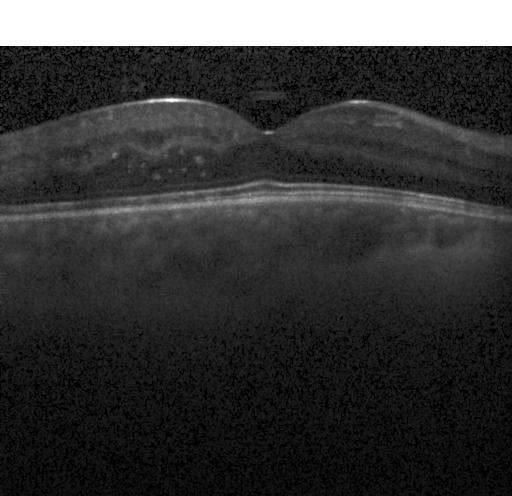

Spectral-domain optical coherence tomography · retinal OCT cross-section · acquired on a Heidelberg Spectralis.
Dx: diabetic macular edema.